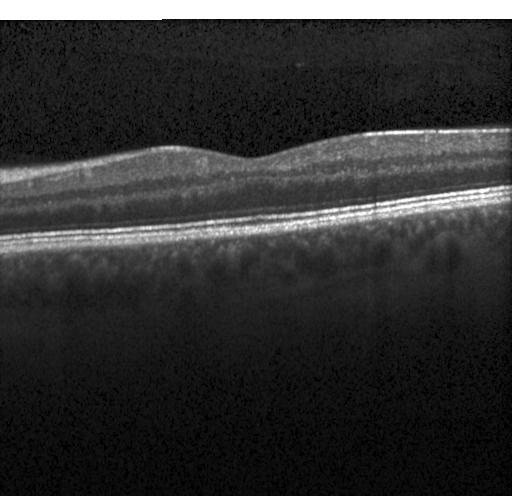

Optical coherence tomography scan; centered on the fovea.
OCT finding: no choroidal neovascularization, diabetic macular edema, or drusen.